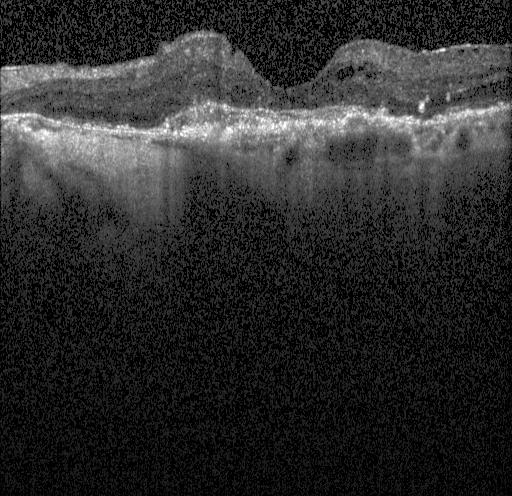

Spectral-domain OCT B-scan: a choroidal neovascular membrane.